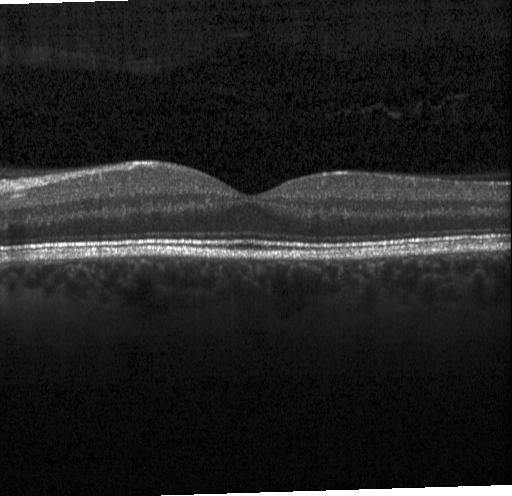
SD-OCT. Through the macula. Optical coherence tomography scan
Impression: neither CNV, DME, nor drusen.